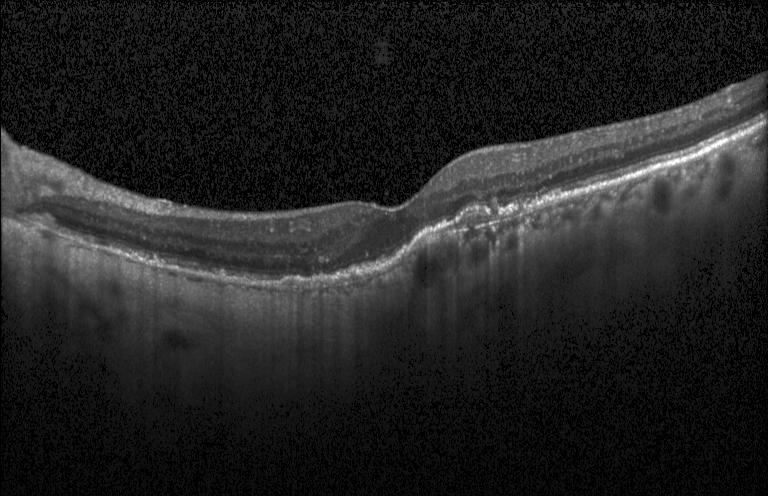 Macular OCT demonstrating a choroidal neovascular membrane.